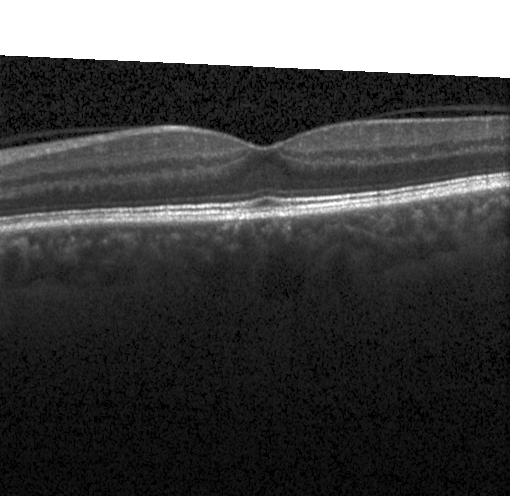
Assessment: no evidence of CNV, DME, or drusen.